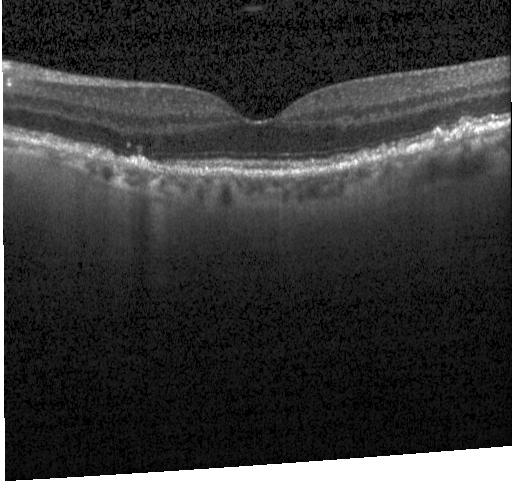

OCT line scan.
Impression: drusen.